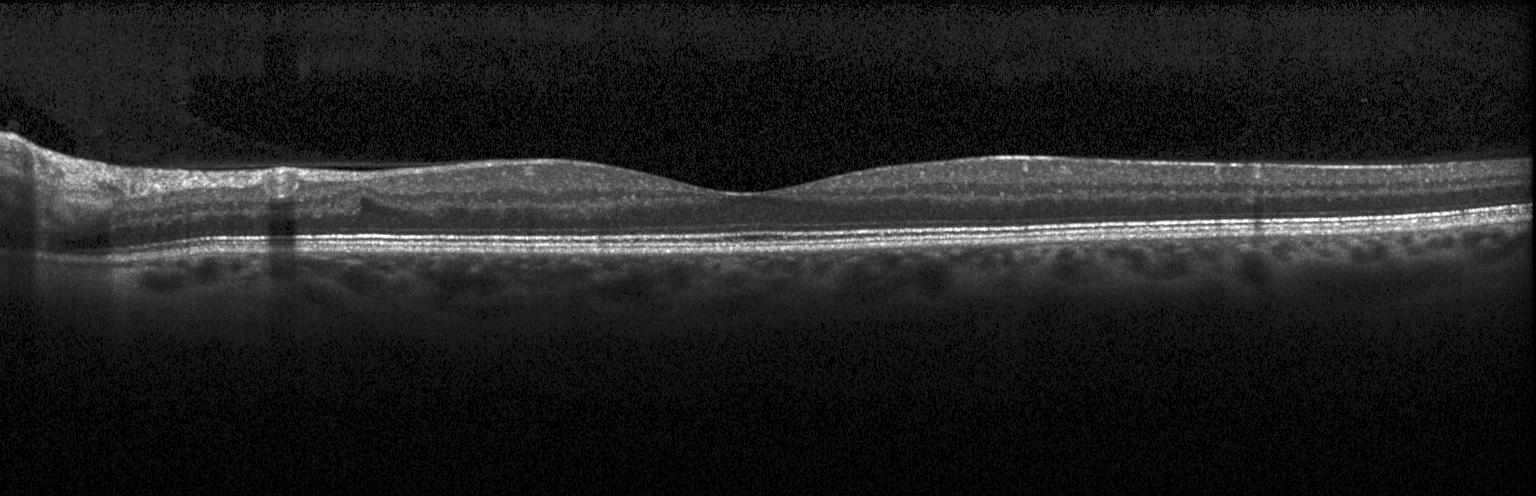

Centered on the fovea. Heidelberg Spectralis OCT system. Spectral-domain OCT. OCT line scan.
Finding: no choroidal neovascularization, no diabetic macular edema, and no drusen.